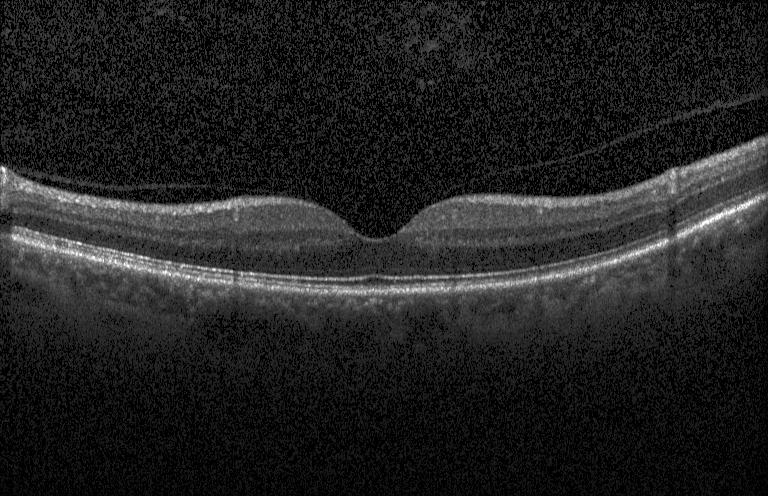 Finding: no CNV, DME, or drusen.